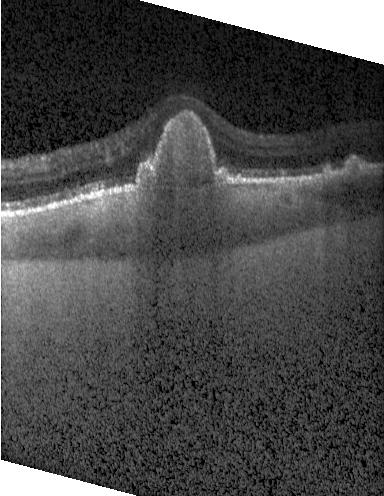 Acquired on a Heidelberg Spectralis. Optical coherence tomography B-scan. Macular scan — Impression: choroidal neovascularization.